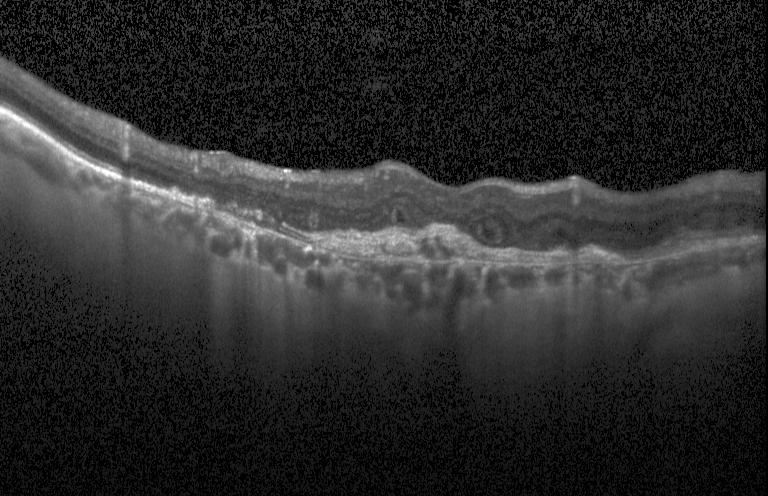
OCT B-scan — Macular OCT: choroidal neovascularization (CNV).